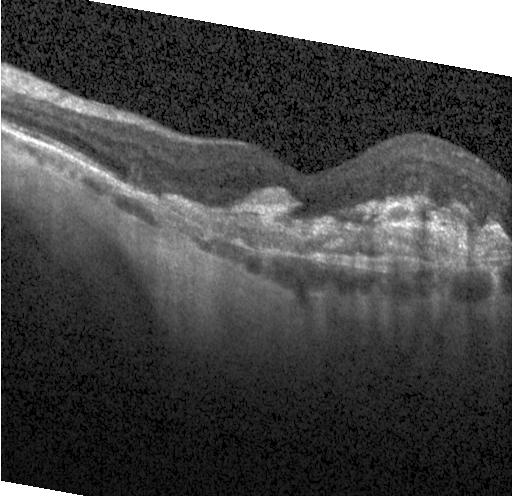
SD-OCT, OCT line scan — Diagnosis: choroidal neovascularization.